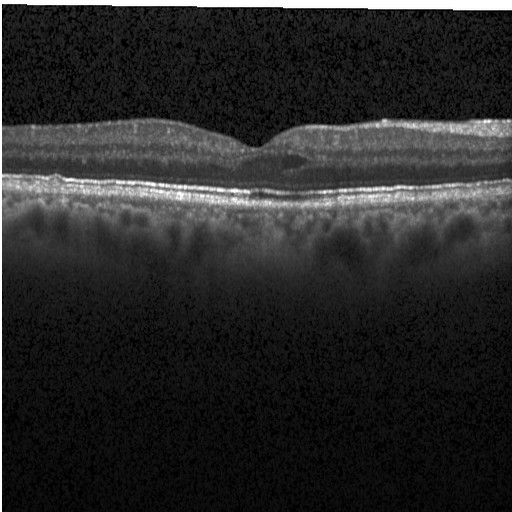

SD-OCT, optical coherence tomography B-scan — OCT finding: diabetic macular edema (DME).